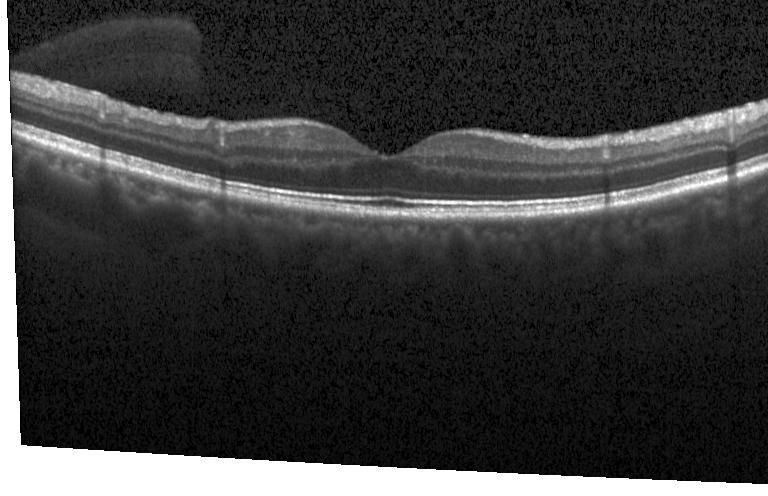

OCT line scan — OCT finding: no evidence of choroidal neovascularization, diabetic macular edema, or drusen.